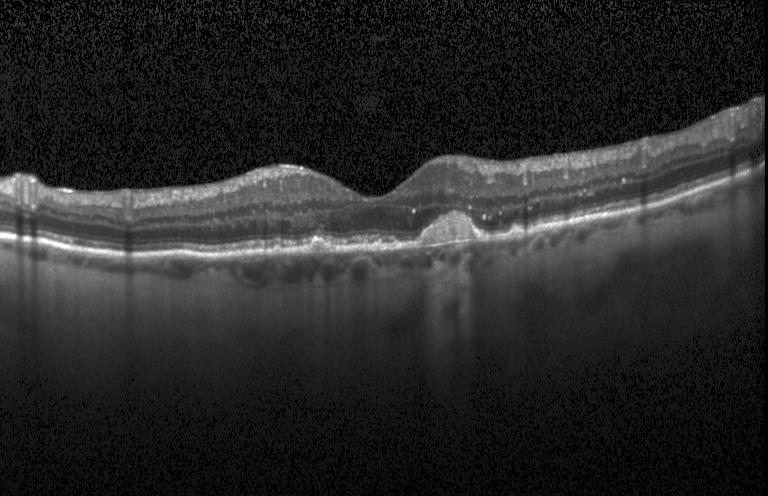
Retinal OCT cross-section showing drusen.